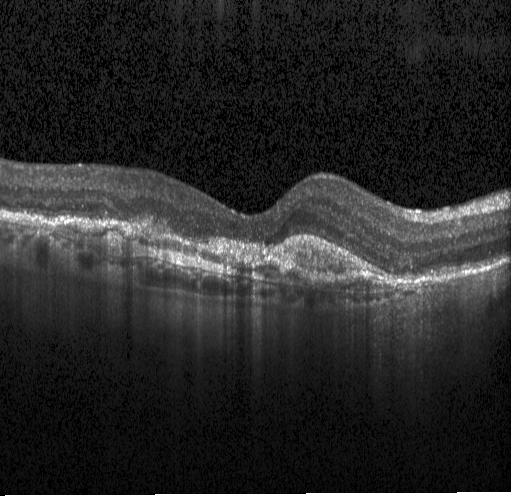 Impression: a choroidal neovascular membrane.